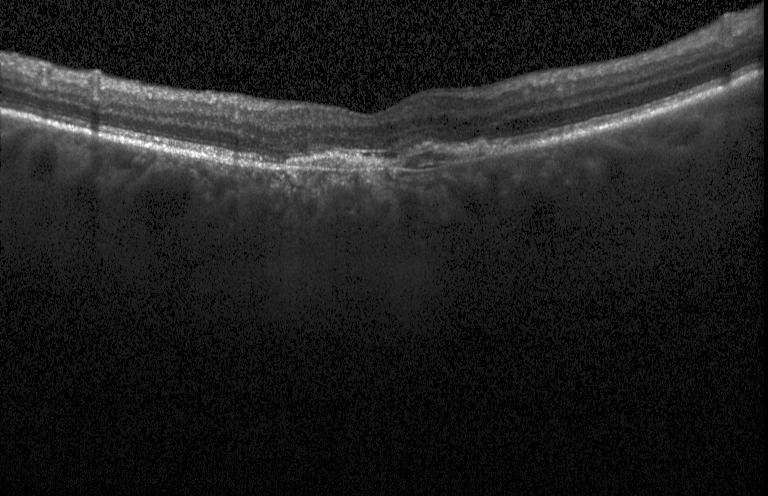
Finding: choroidal neovascularization (CNV).